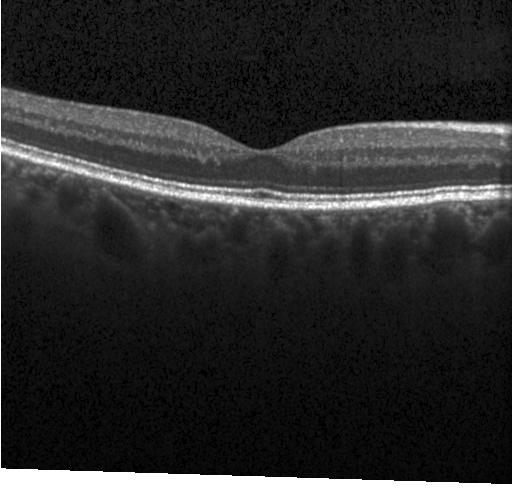

Dx: no CNV, no DME, and no drusen.